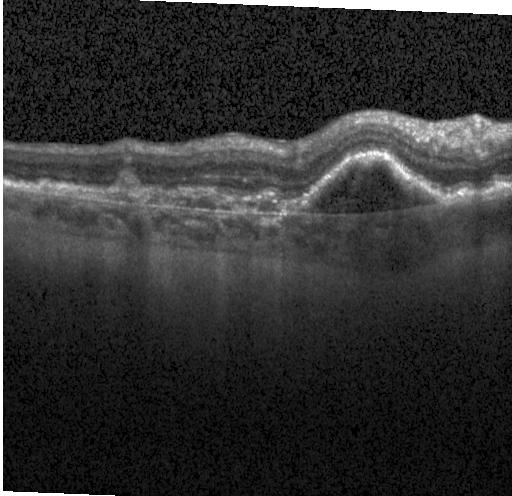

Finding: choroidal neovascularization (CNV).